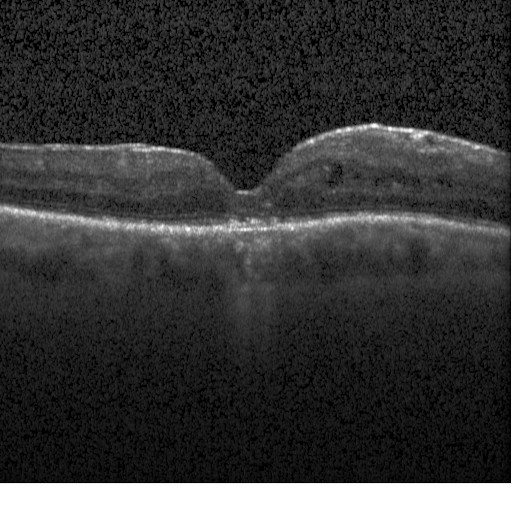
The scan shows diabetic macular edema.